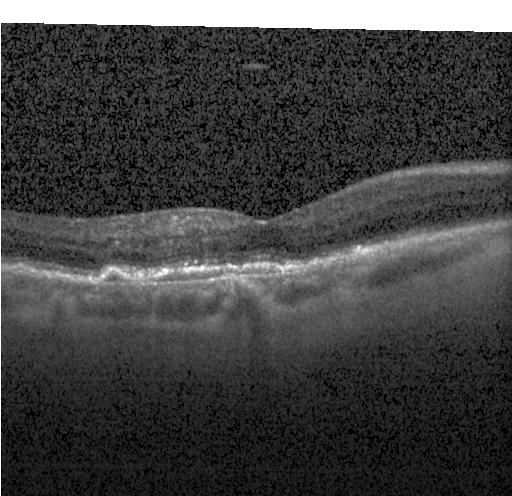 Fovea-centered · OCT B-scan · spectral-domain optical coherence tomography
The scan shows CNV.